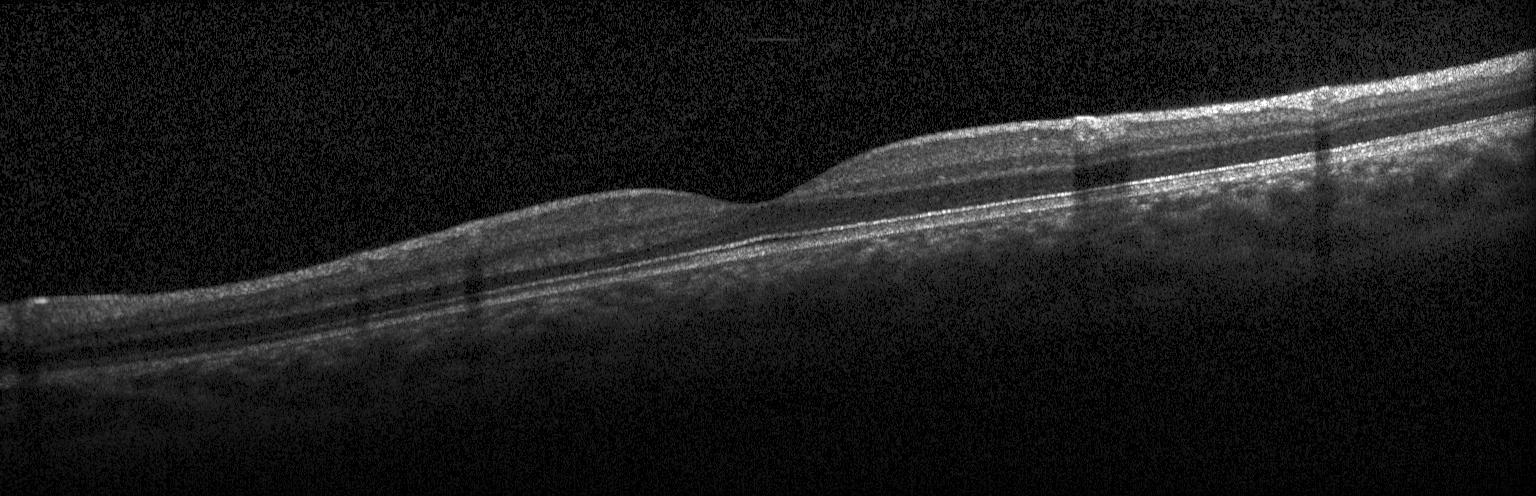 Spectral-domain OCT B-scan: no choroidal neovascularization, no diabetic macular edema, and no drusen.